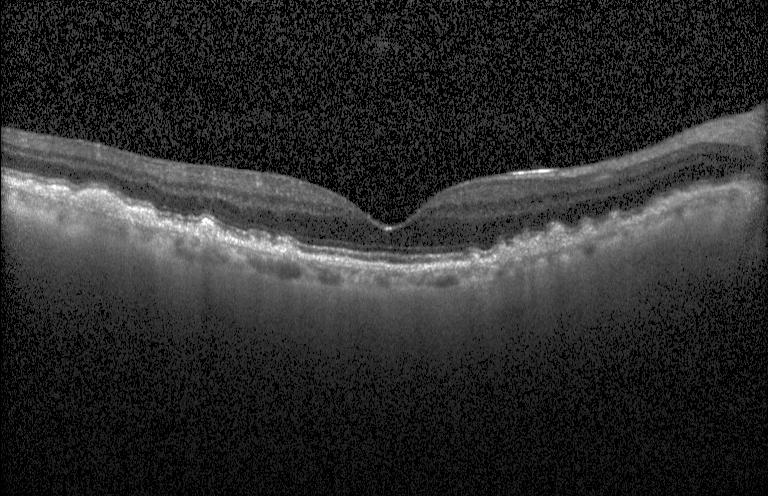
OCT B-scan showing drusen.